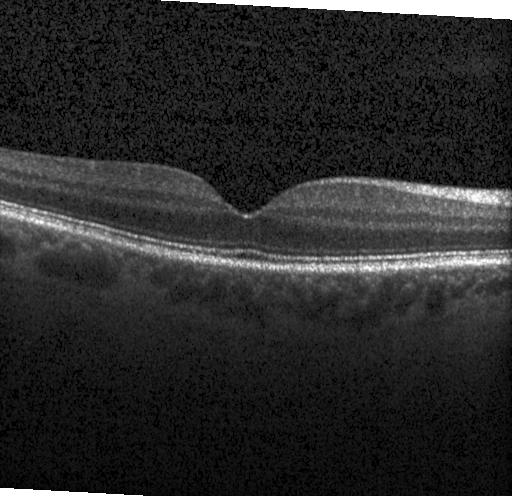
OCT line scan, SD-OCT.
Impression: no CNV, no DME, and no drusen.